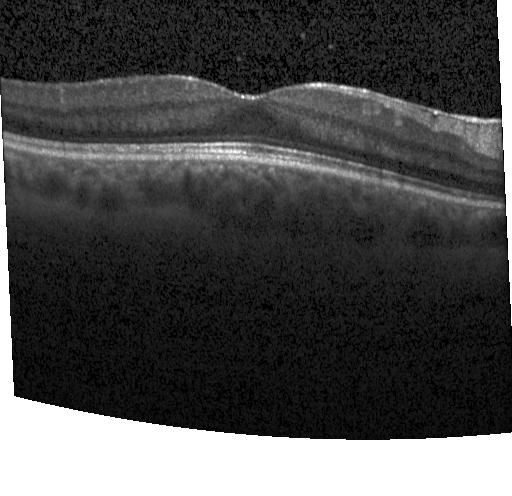
OCT finding: no choroidal neovascularization, no diabetic macular edema, and no drusen.